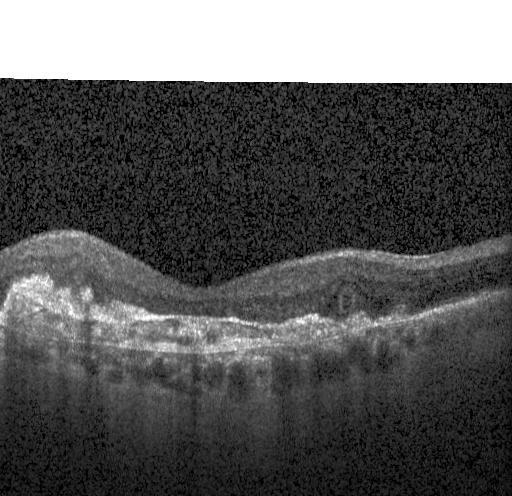 Spectral-domain optical coherence tomography; OCT B-scan. A choroidal neovascular membrane.